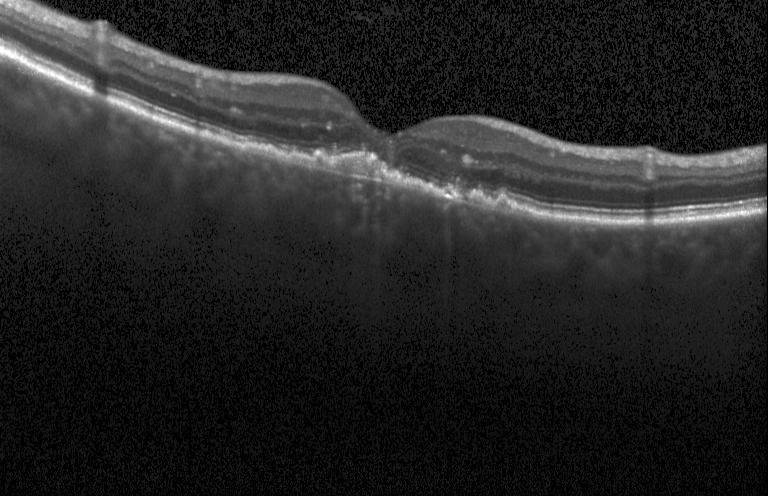
Dx: a choroidal neovascular membrane.